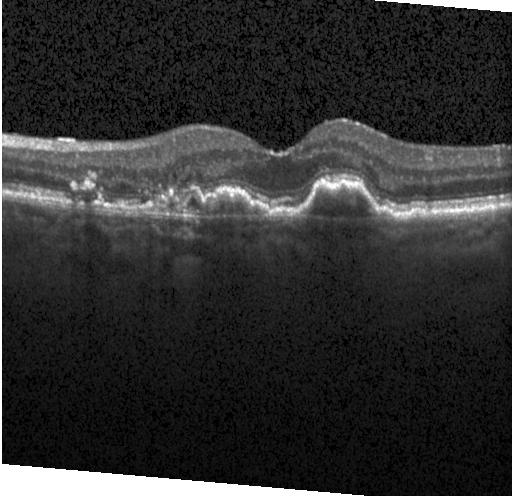
OCT line scan. Dx: a choroidal neovascular membrane.